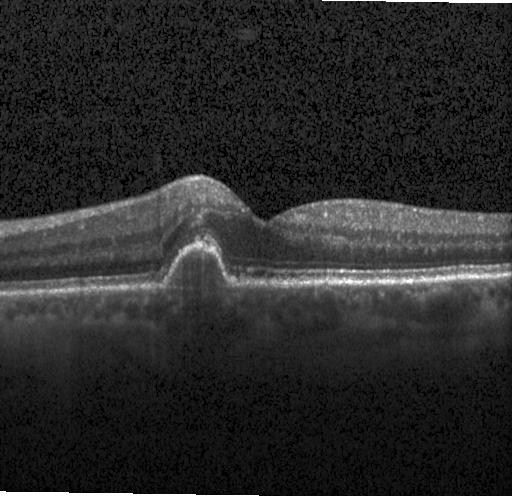

Retinal OCT cross-section.
The scan shows a choroidal neovascular membrane.